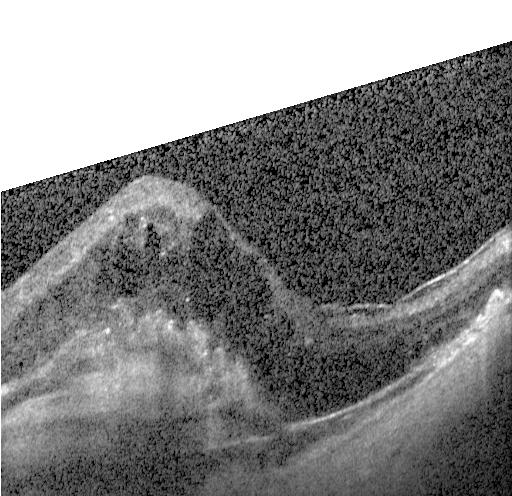

Centered on the fovea; optical coherence tomography B-scan; Heidelberg Spectralis — Macular OCT: a choroidal neovascular membrane.